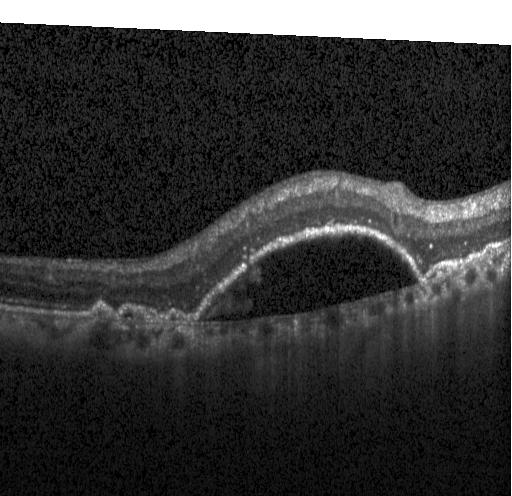 Retinal OCT B-scan; fovea-centered. Diagnosis: a choroidal neovascular membrane.